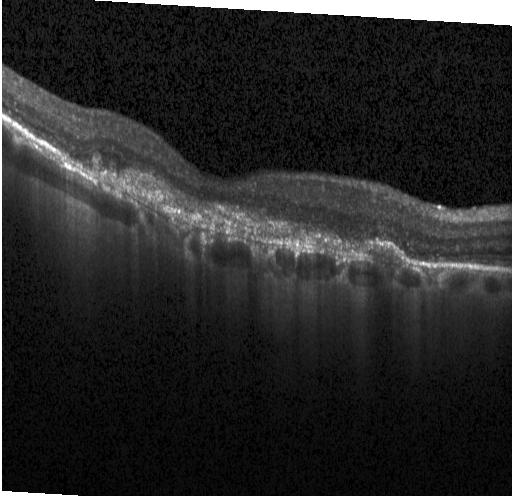

Retinal OCT cross-section. SD-OCT. Horizontal scan through the fovea
Finding: a choroidal neovascular membrane.